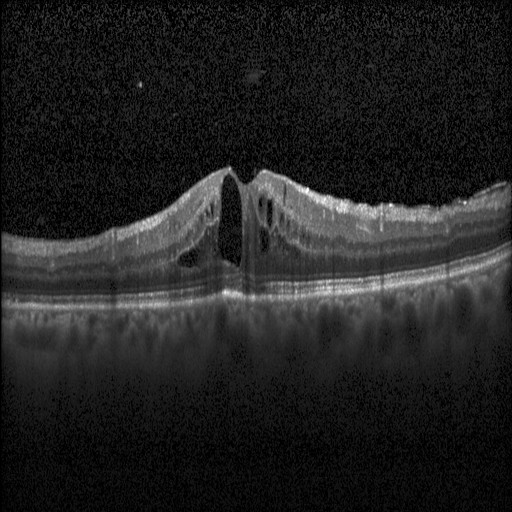
OCT B-scan — OCT finding: diabetic macular edema.